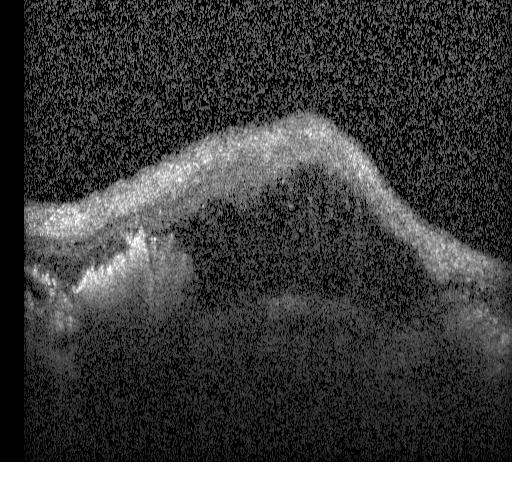

Impression: diabetic macular edema (DME).